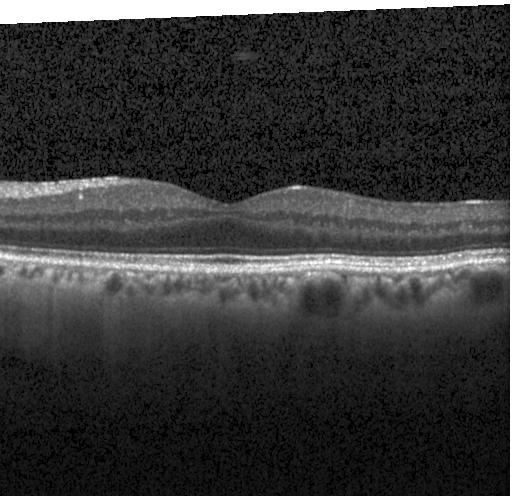

SD-OCT. OCT line scan. Heidelberg Spectralis. This B-scan demonstrates no choroidal neovascularization, no diabetic macular edema, and no drusen.